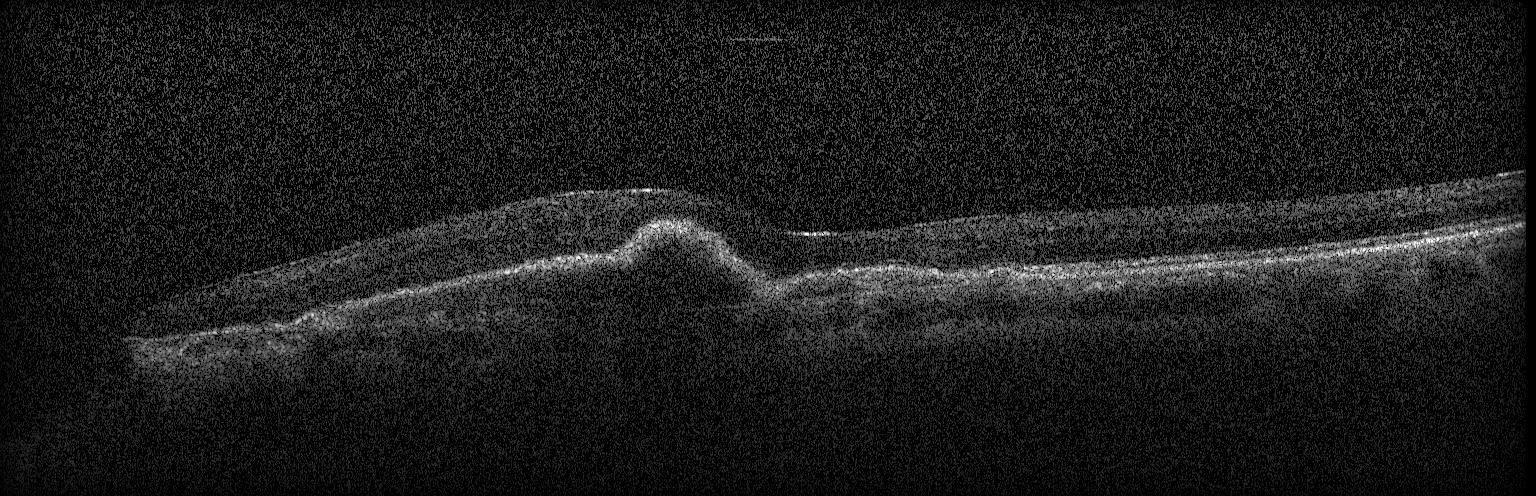
Spectral-domain OCT B-scan: choroidal neovascularization.